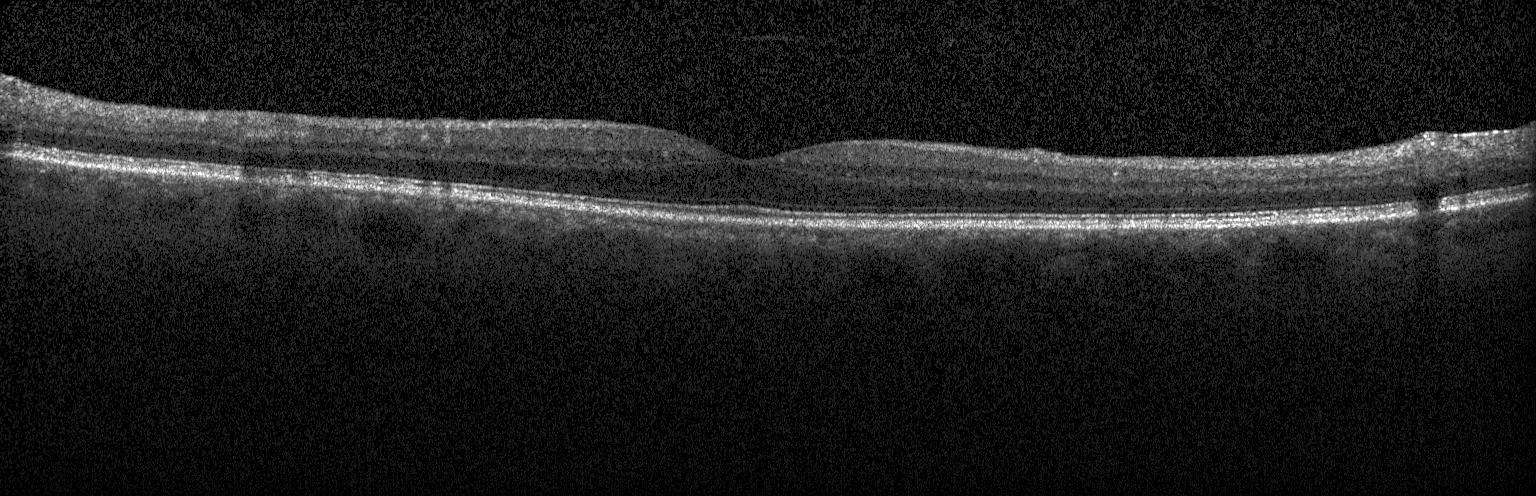
Impression: no choroidal neovascularization, no diabetic macular edema, and no drusen.